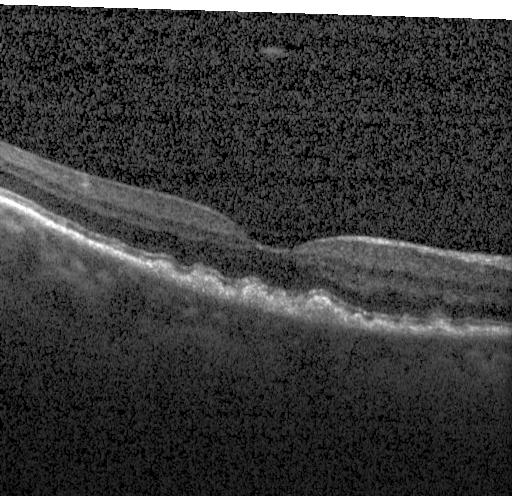

Acquired on a Heidelberg Spectralis, optical coherence tomography B-scan, macular scan — OCT finding: sub-RPE drusenoid deposits.